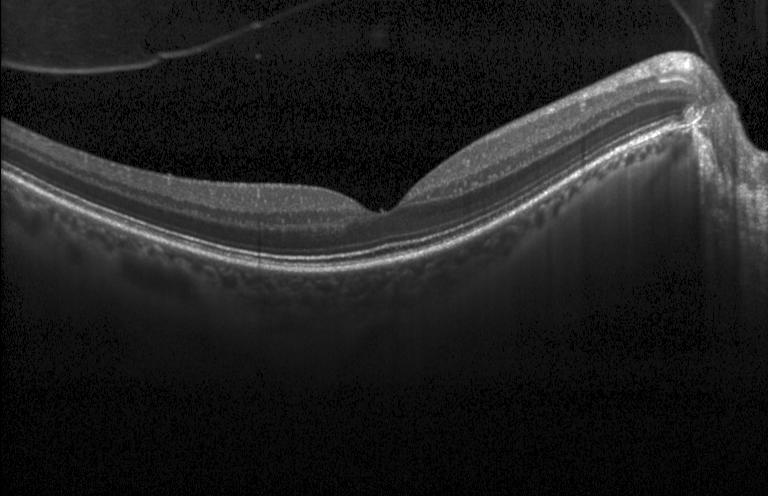
Dx: no evidence of choroidal neovascularization, diabetic macular edema, or drusen.